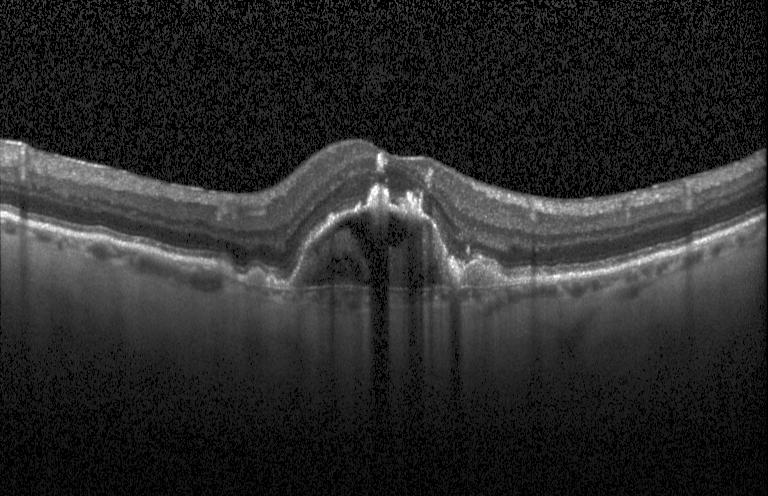
Diagnosis: choroidal neovascularization.